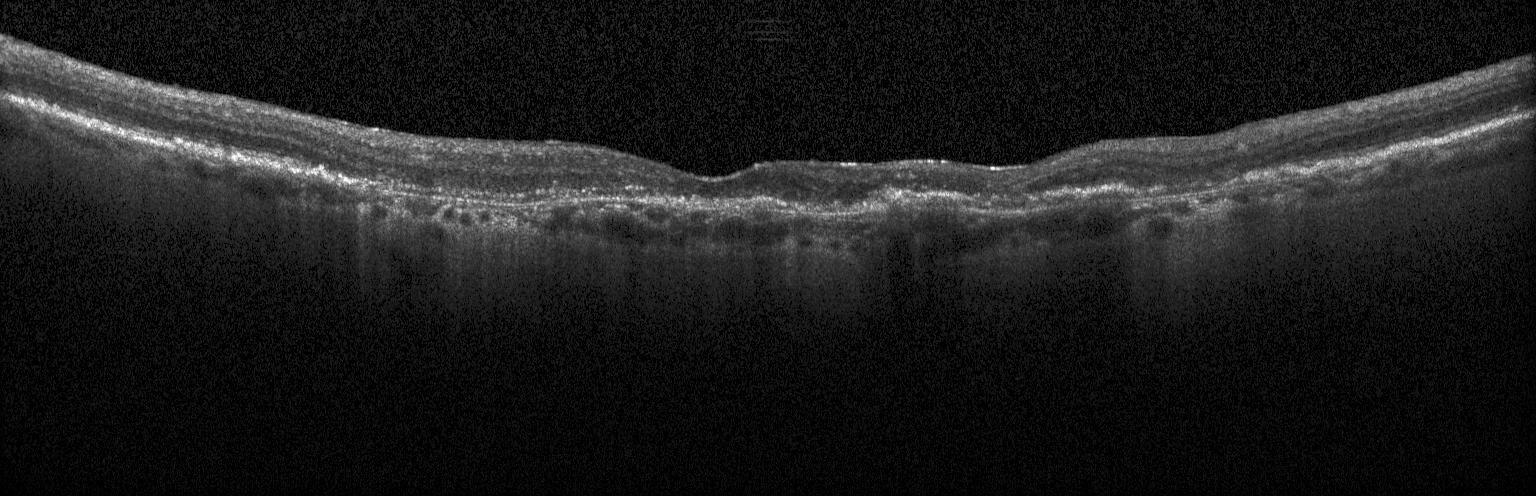

Macular OCT: a choroidal neovascular membrane.